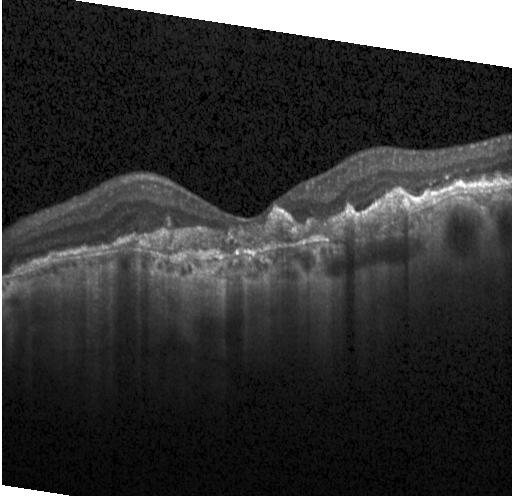
OCT B-scan; Heidelberg Spectralis OCT system.
A choroidal neovascular membrane.